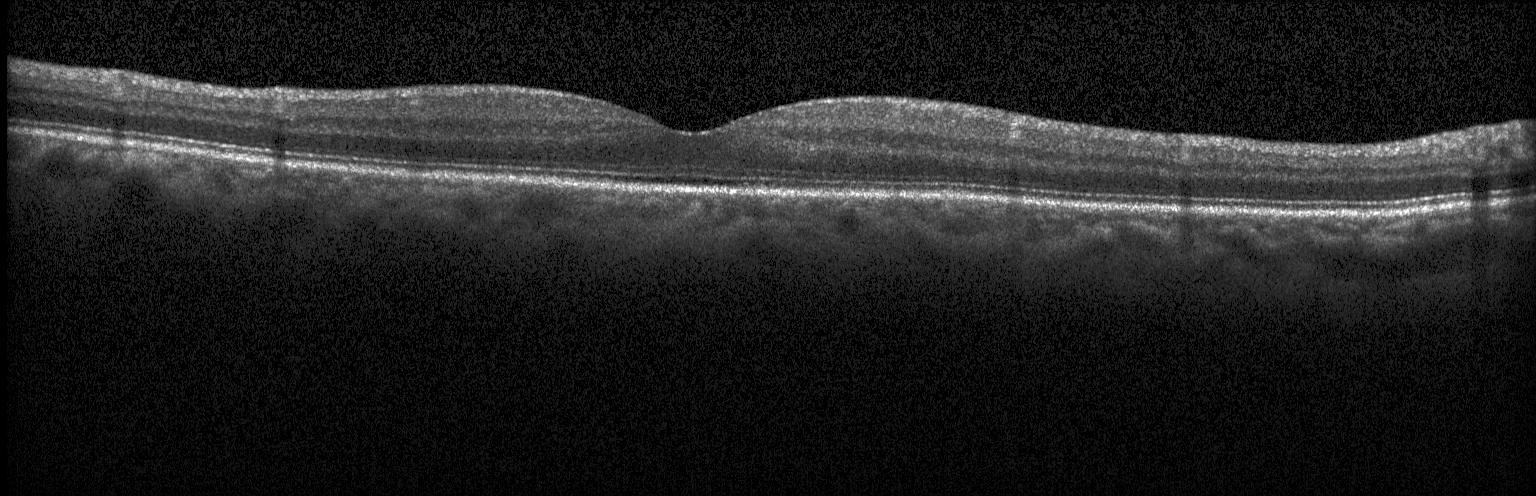
Retinal OCT cross-section showing no choroidal neovascularization, diabetic macular edema, or drusen.